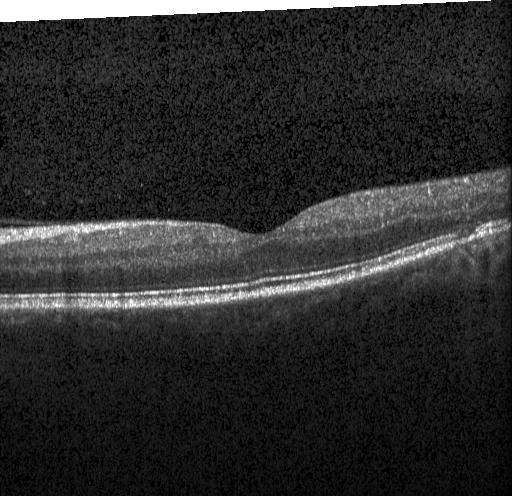
Optical coherence tomography B-scan, fovea-centered, Heidelberg Spectralis OCT system. The scan shows no choroidal neovascularization, diabetic macular edema, or drusen.